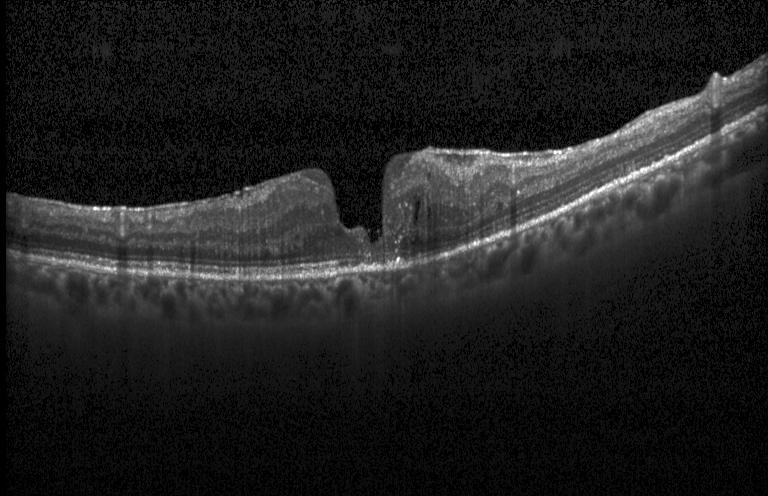 Retinal OCT B-scan.
Diagnosis: diabetic macular edema (DME).